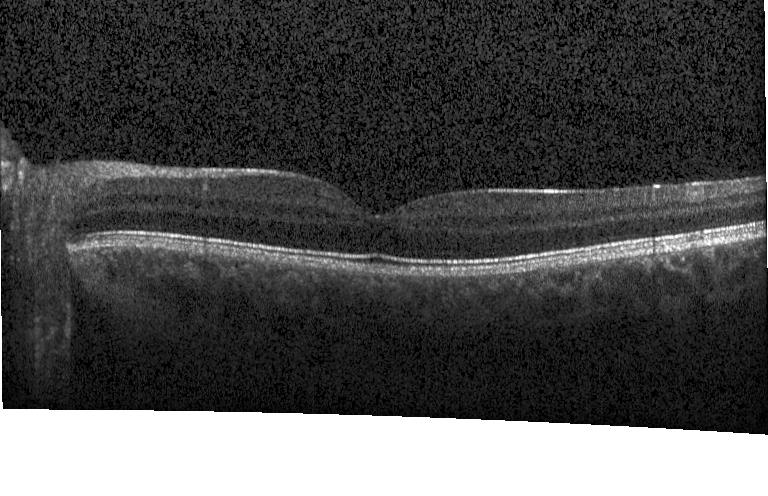
SD-OCT. Centered on the fovea. Optical coherence tomography B-scan. Acquired on a Heidelberg Spectralis.
Impression: no evidence of choroidal neovascularization, diabetic macular edema, or drusen.